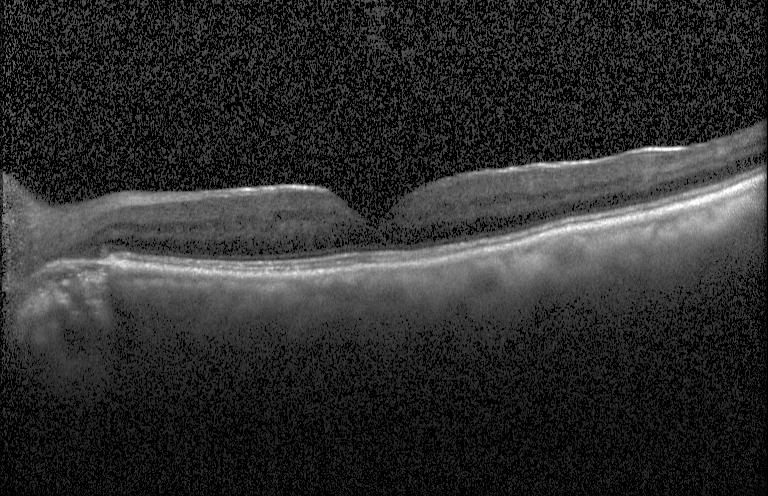 OCT finding: no choroidal neovascularization, diabetic macular edema, or drusen.